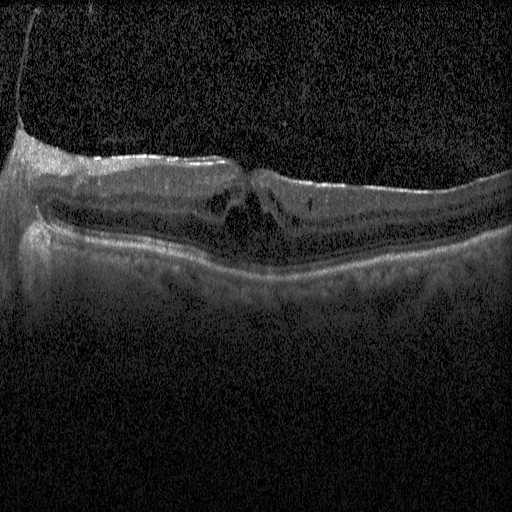 OCT line scan · macular scan — This B-scan demonstrates diabetic macular edema (DME).